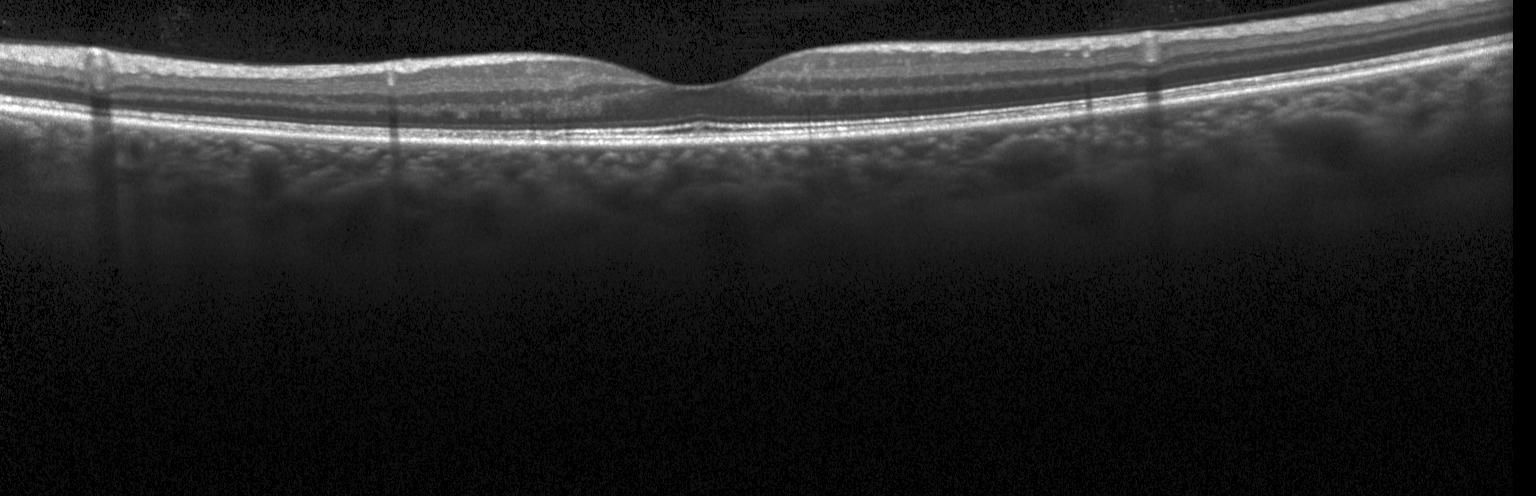

SD-OCT, OCT B-scan.
Finding: no evidence of CNV, DME, or drusen.